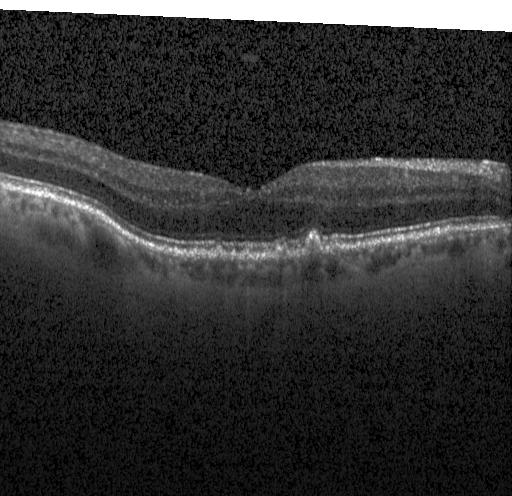
Multiple drusen.